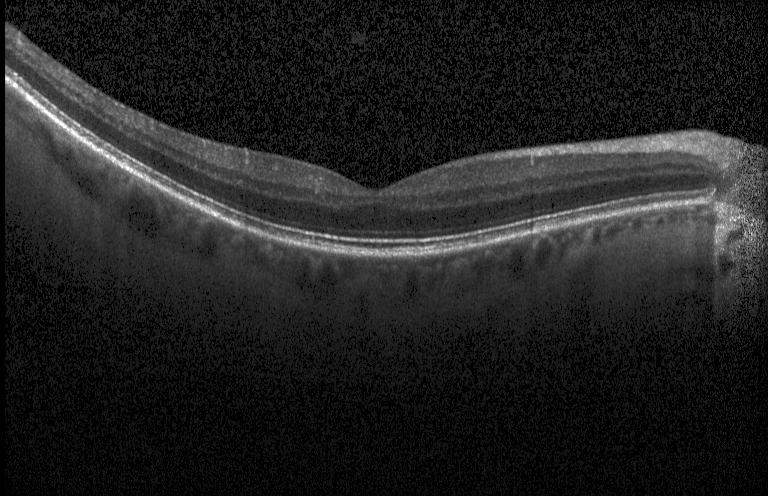

This B-scan demonstrates no choroidal neovascularization, no diabetic macular edema, and no drusen.